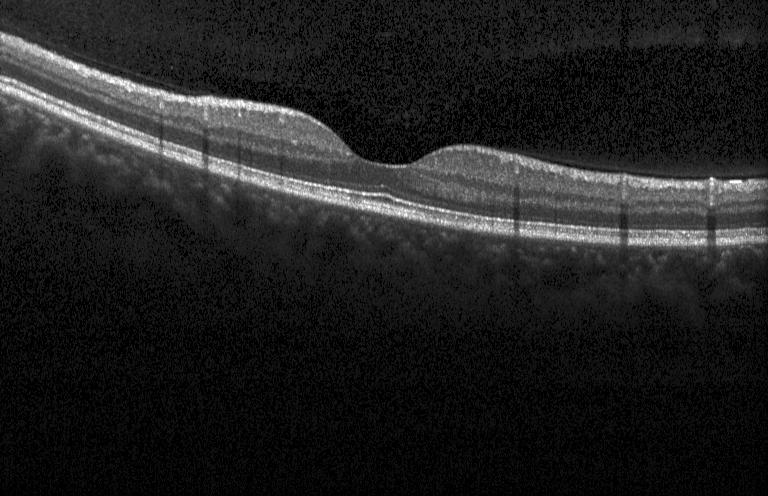

Macular OCT demonstrating no choroidal neovascularization, diabetic macular edema, or drusen.